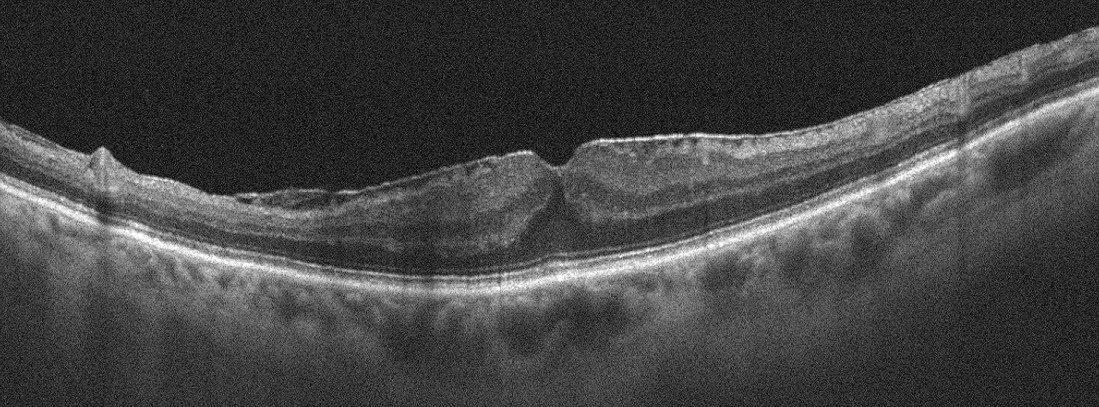
Retinal OCT cross-section. Macular scan.
Assessment: ERM.